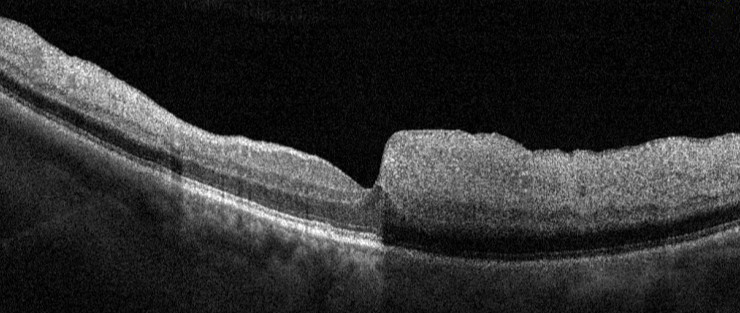

OCT B-scan showing retinal artery occlusion.